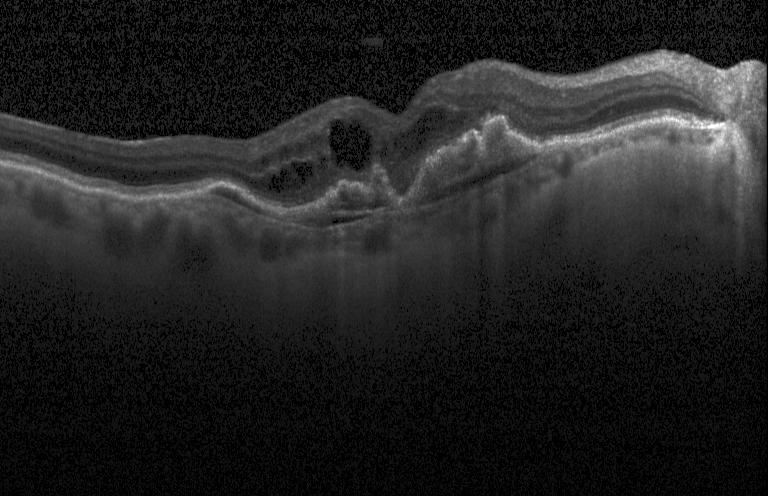

Optical coherence tomography scan; instrument: Heidelberg Spectralis; spectral-domain OCT; fovea-centered
The scan shows a choroidal neovascular membrane.